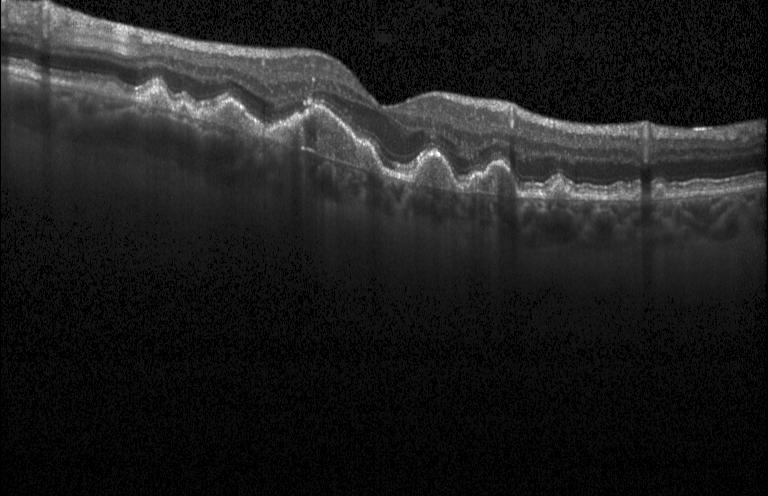
Spectral-domain OCT B-scan: multiple drusen.